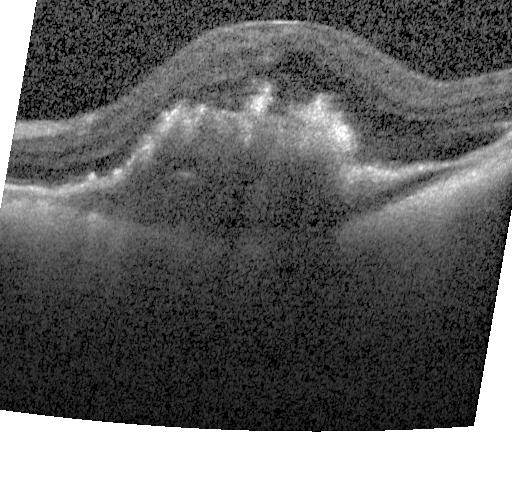 Fovea-centered; spectral-domain OCT; Heidelberg Spectralis; retinal OCT cross-section — Impression: a choroidal neovascular membrane.